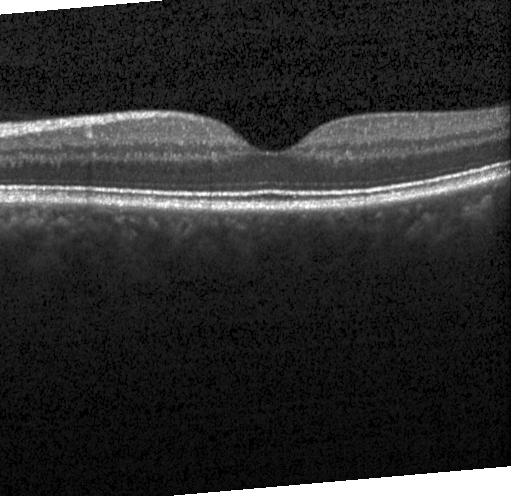 OCT B-scan; Heidelberg Spectralis; through the macula — Diagnosis: no evidence of choroidal neovascularization, diabetic macular edema, or drusen.